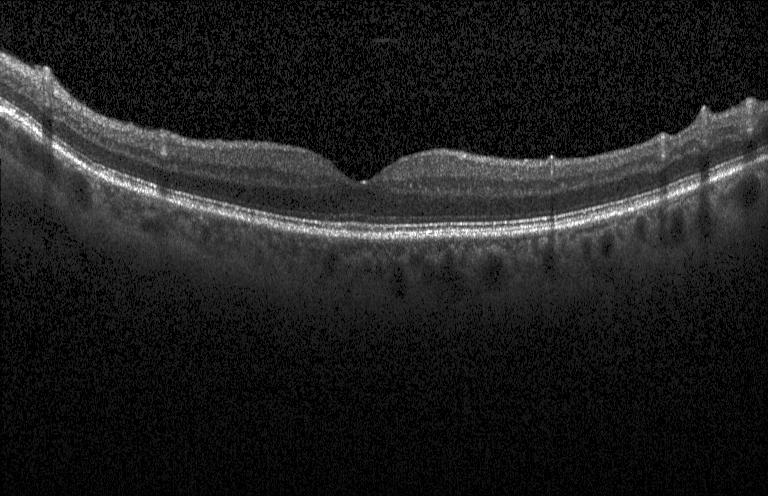

Optical coherence tomography B-scan. Spectral-domain optical coherence tomography. Through the macula — Impression: no CNV, DME, or drusen.